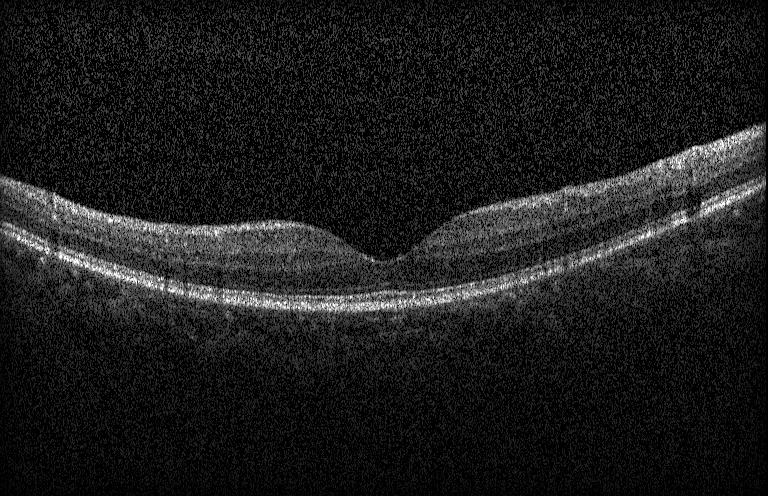 Impression: no choroidal neovascularization, diabetic macular edema, or drusen.